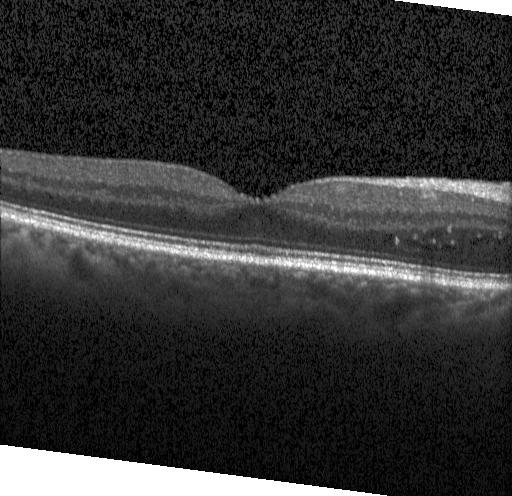

Acquired on a Heidelberg Spectralis. Retinal OCT B-scan. Spectral-domain optical coherence tomography.
Finding: no evidence of choroidal neovascularization, diabetic macular edema, or drusen.